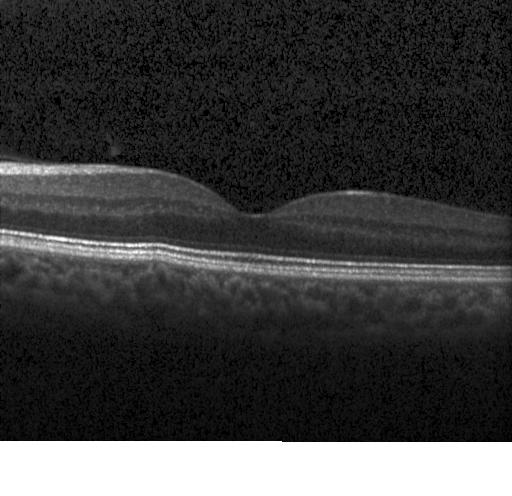
Retinal OCT cross-section — OCT finding: no choroidal neovascularization, diabetic macular edema, or drusen.